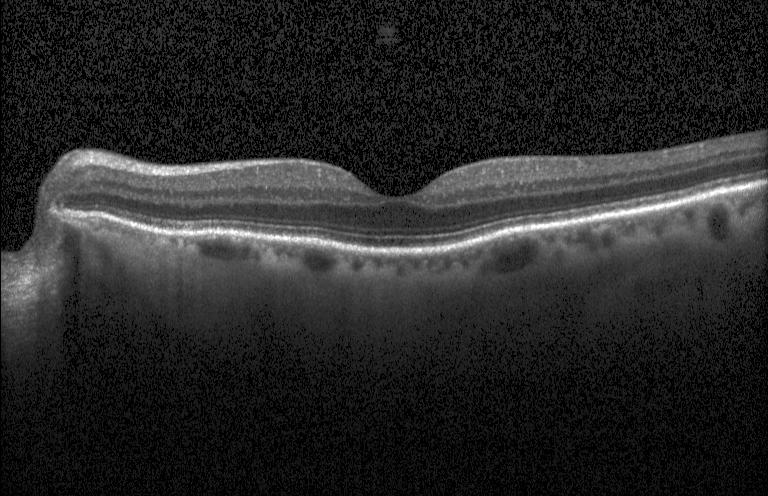 OCT B-scan · spectral-domain OCT
Diagnosis: neither choroidal neovascularization, diabetic macular edema, nor drusen.